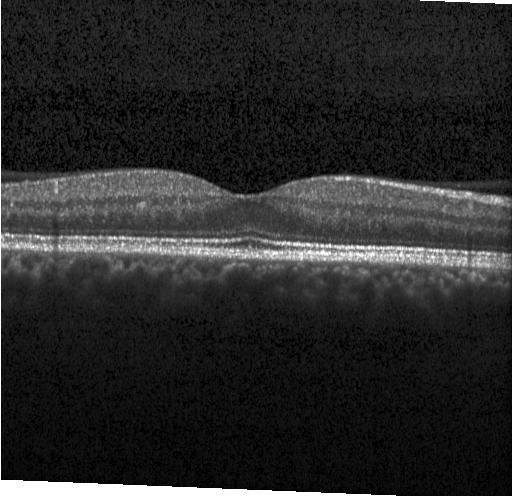

OCT B-scan showing no choroidal neovascularization, diabetic macular edema, or drusen.